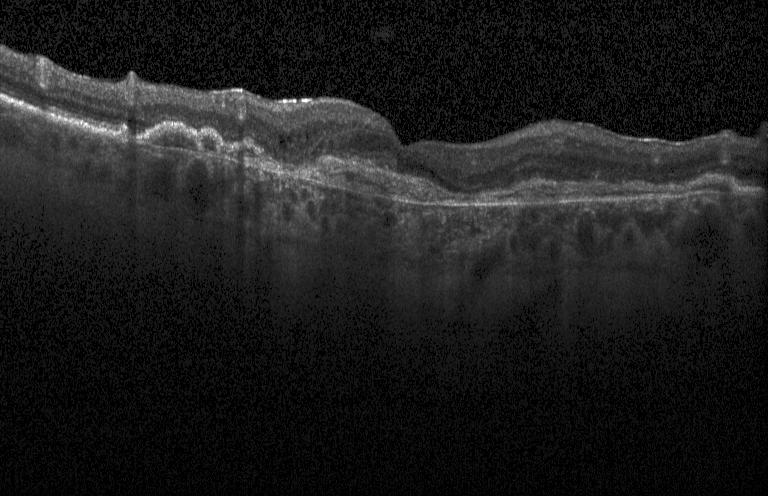
OCT line scan. Centered on the fovea. Spectral-domain OCT. Instrument: Heidelberg Spectralis
Dx: a choroidal neovascular membrane.